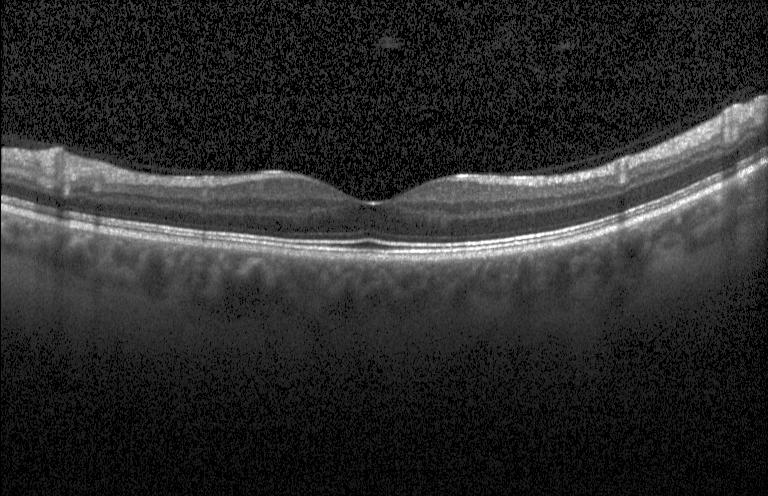
No choroidal neovascularization, no diabetic macular edema, and no drusen.